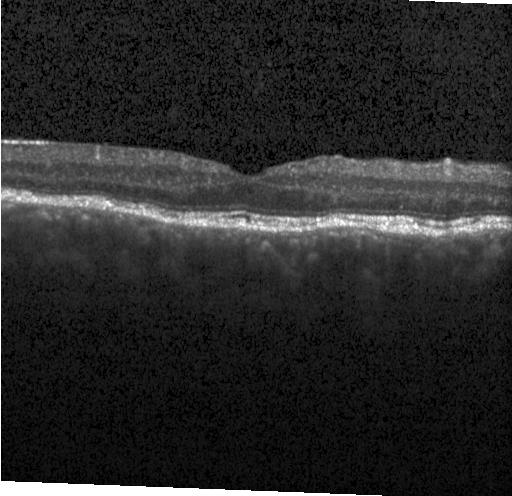 Finding: no evidence of choroidal neovascularization, diabetic macular edema, or drusen.